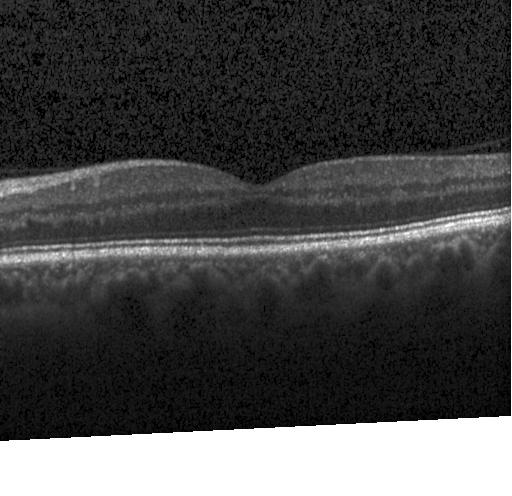 Spectral-domain optical coherence tomography. Heidelberg Spectralis OCT system. Through the macula. Optical coherence tomography B-scan. OCT finding: no choroidal neovascularization, diabetic macular edema, or drusen.